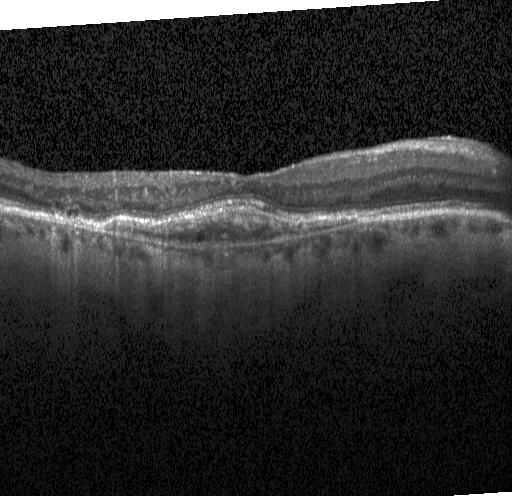 Retinal OCT B-scan, centered on the fovea, acquired on a Heidelberg Spectralis, spectral-domain OCT. Macular OCT: a choroidal neovascular membrane.